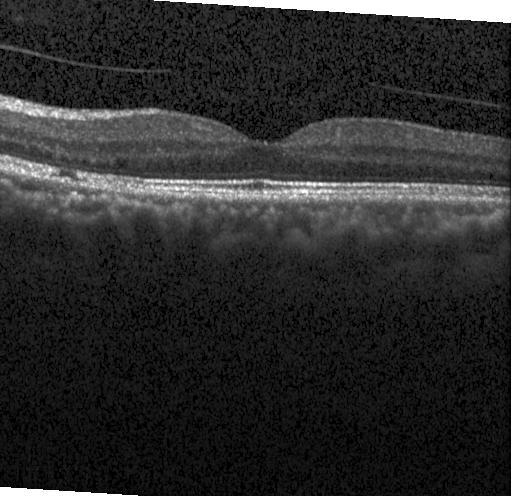
Retinal OCT cross-section · acquired on a Heidelberg Spectralis · spectral-domain optical coherence tomography
Diagnosis: no choroidal neovascularization, diabetic macular edema, or drusen.